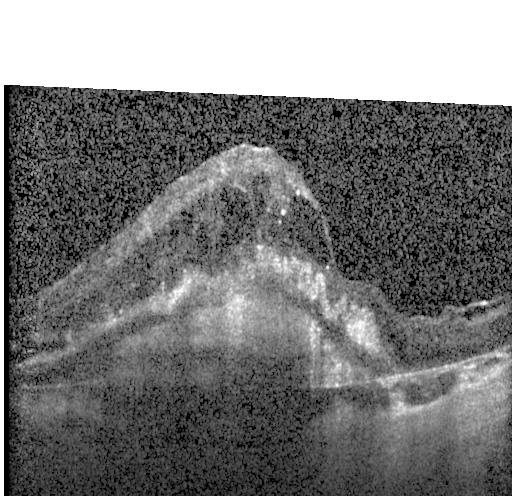 OCT B-scan — Diagnosis: choroidal neovascularization.